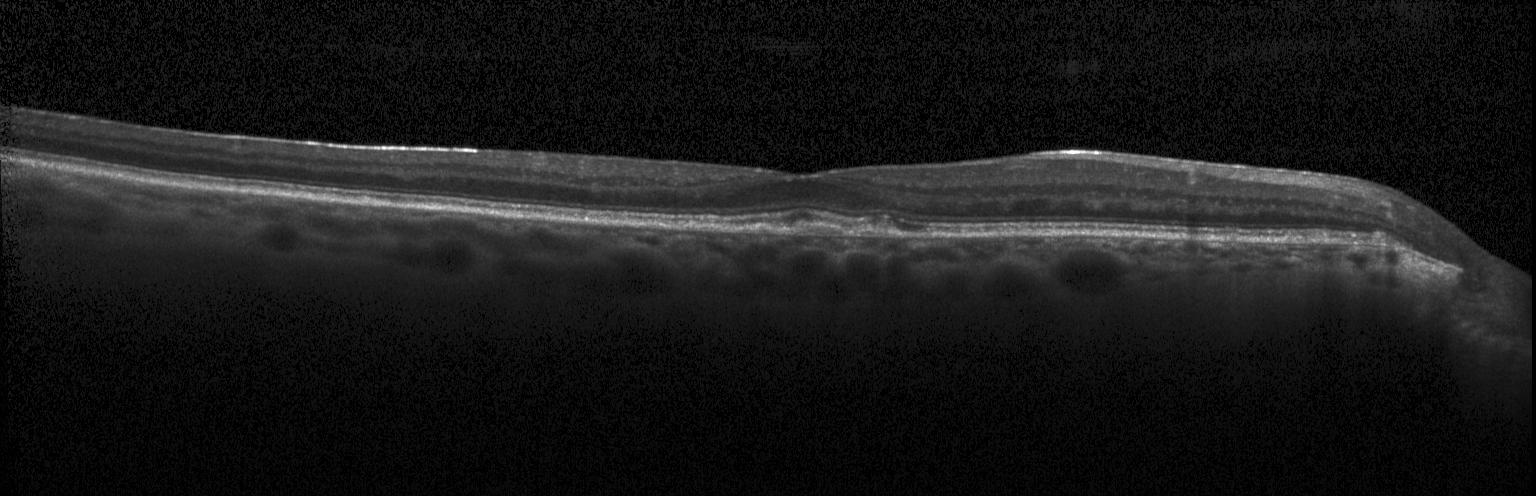

Spectral-domain OCT B-scan: sub-RPE drusenoid deposits.